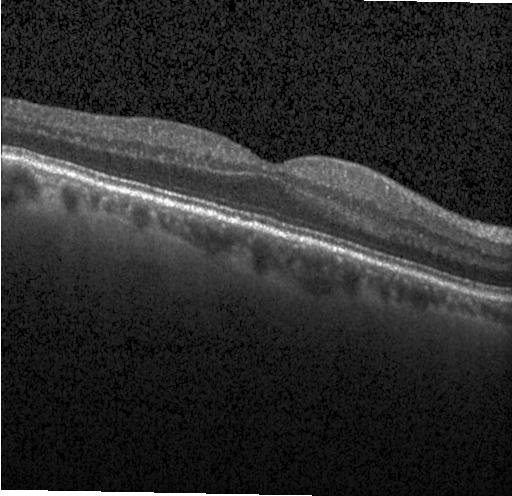
Retinal OCT B-scan. Heidelberg Spectralis
This B-scan demonstrates no evidence of CNV, DME, or drusen.